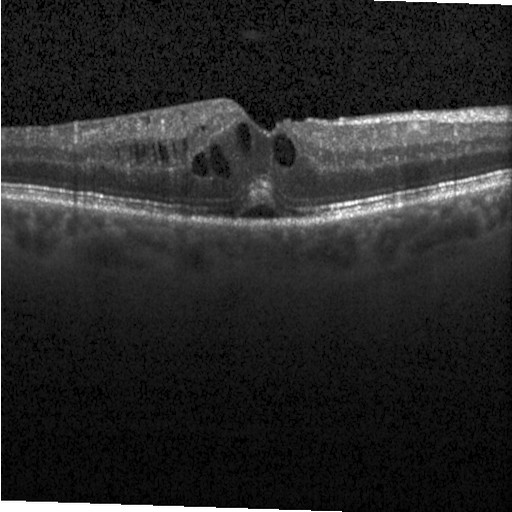
Diagnosis: diabetic macular edema.